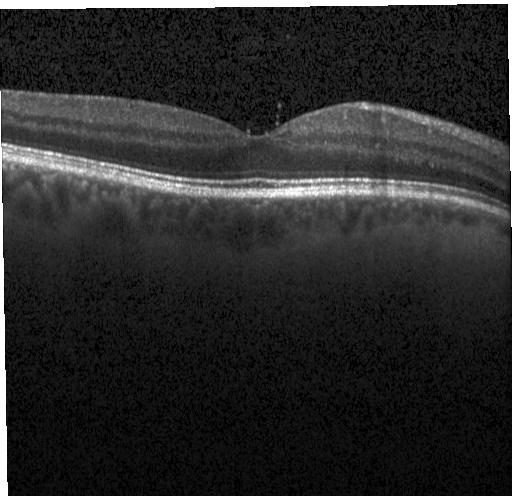
OCT B-scan showing neither choroidal neovascularization, diabetic macular edema, nor drusen.